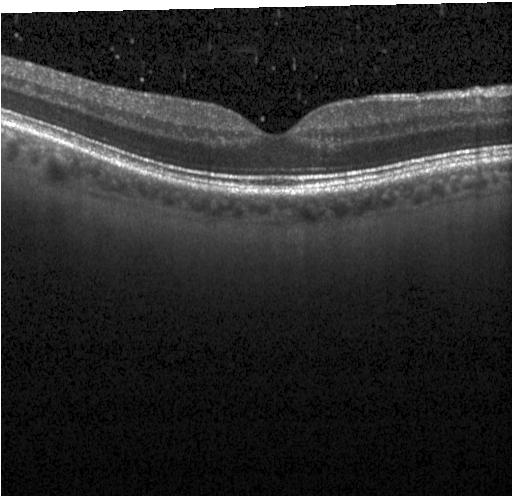
Impression: no evidence of choroidal neovascularization, diabetic macular edema, or drusen.